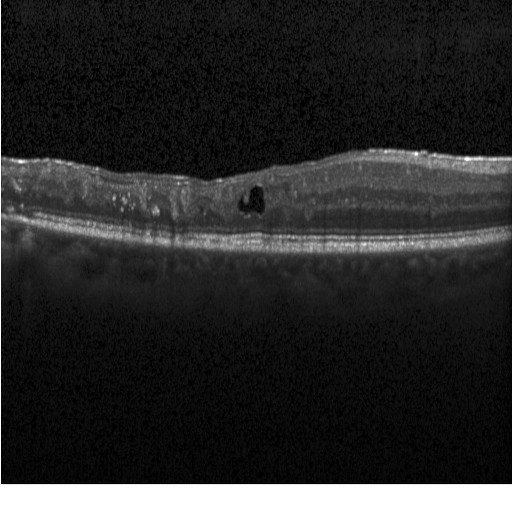
Assessment: DME.